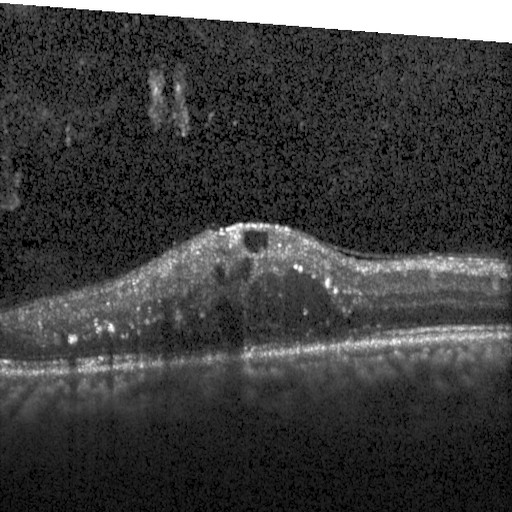 Retinal OCT cross-section — Assessment: diabetic macular edema (DME).